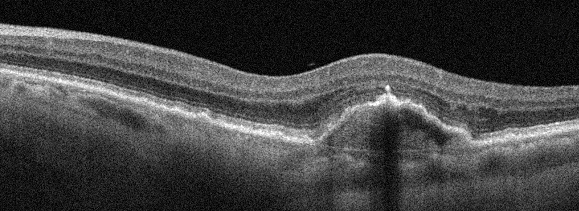 Instrument: Optovue Avanti RTVue XR · through the macula · retinal OCT B-scan — Diagnosis: age-related macular degeneration.